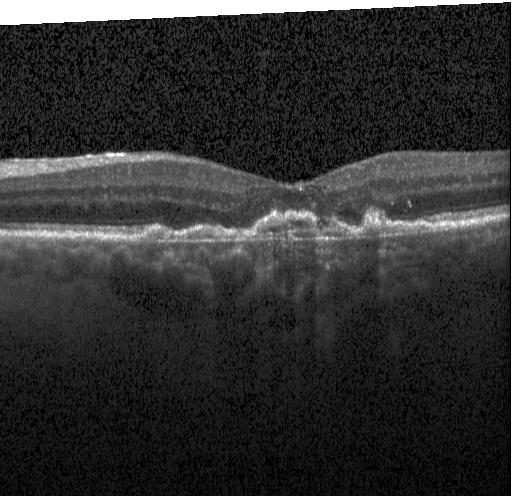 Retinal OCT cross-section.
The scan shows a choroidal neovascular membrane.